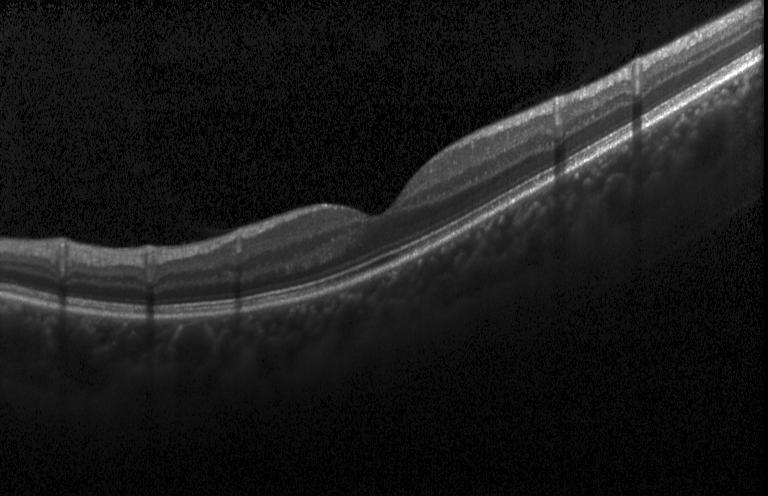

Spectral-domain optical coherence tomography, instrument: Heidelberg Spectralis, macular scan, retinal OCT B-scan — Macular OCT: neither choroidal neovascularization, diabetic macular edema, nor drusen.